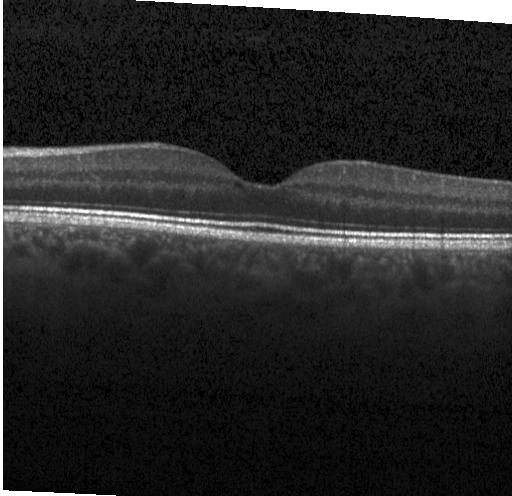
Impression: no evidence of CNV, DME, or drusen.